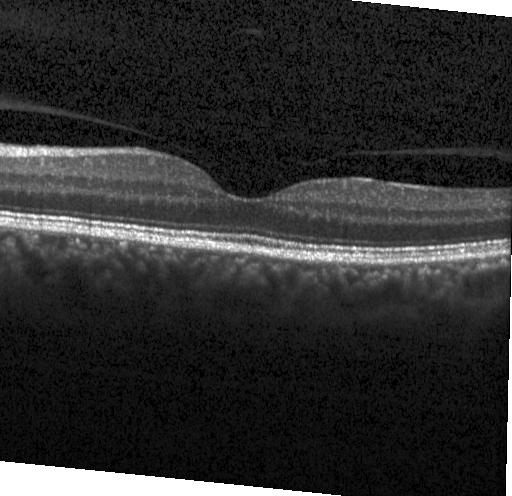
OCT line scan, macular scan.
Impression: neither choroidal neovascularization, diabetic macular edema, nor drusen.